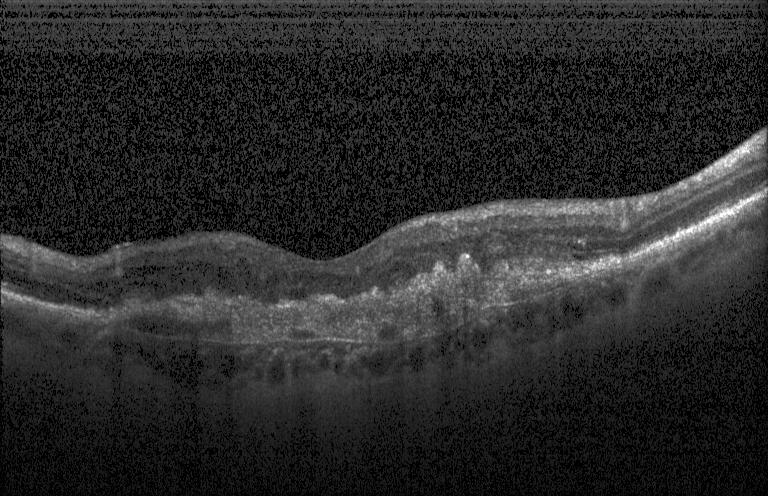
A choroidal neovascular membrane.